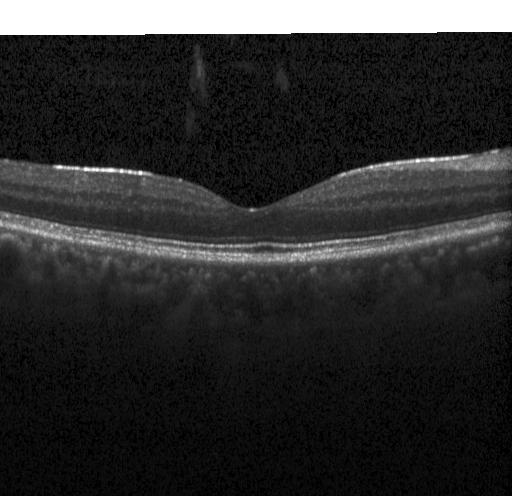
OCT line scan
The scan shows no CNV, DME, or drusen.